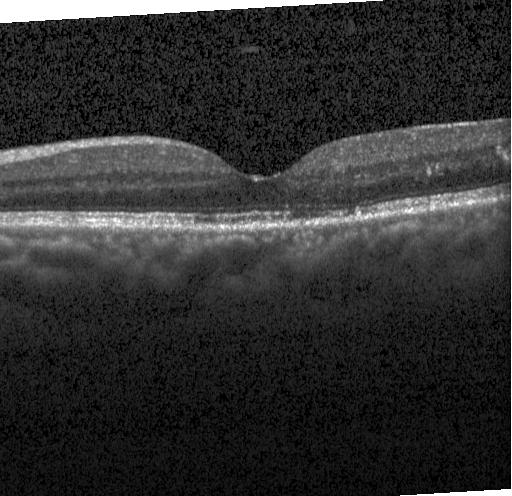 OCT finding: no choroidal neovascularization, diabetic macular edema, or drusen.